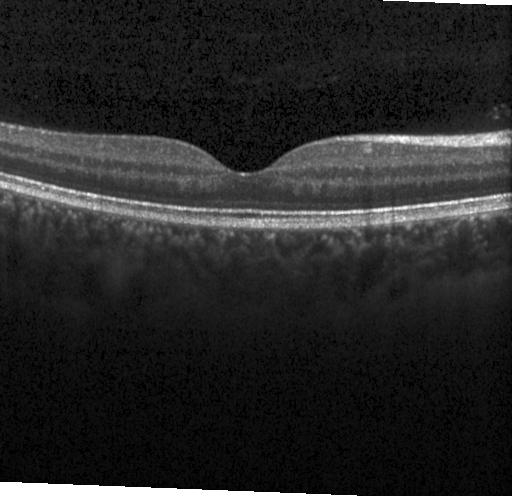 Instrument: Heidelberg Spectralis; OCT line scan. Finding: no evidence of choroidal neovascularization, diabetic macular edema, or drusen.